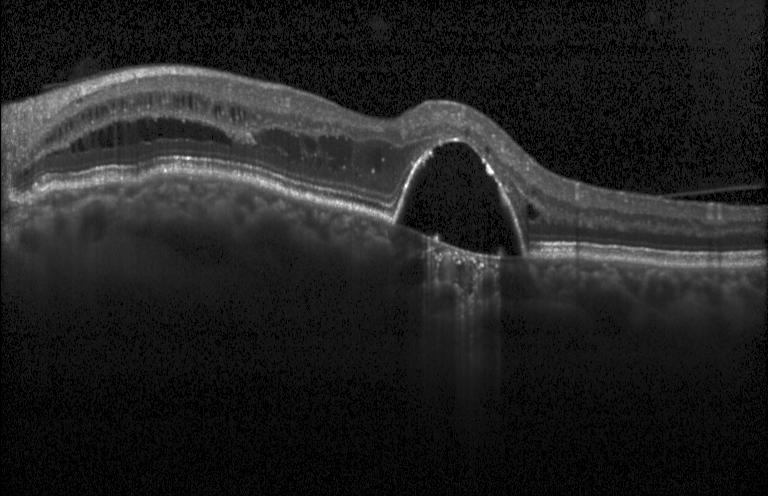
Diagnosis: a choroidal neovascular membrane.